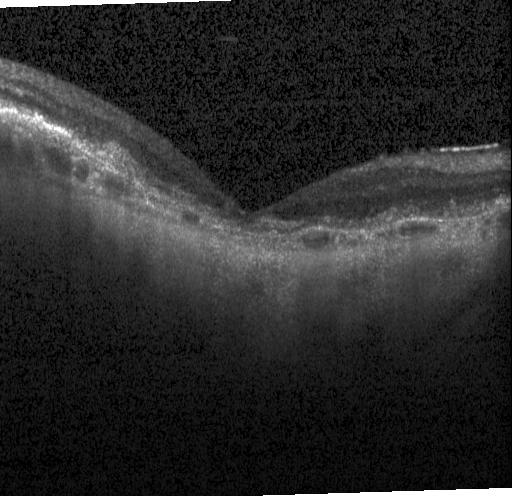 SD-OCT. Acquired on a Heidelberg Spectralis. Centered on the fovea. OCT B-scan — Finding: choroidal neovascularization.